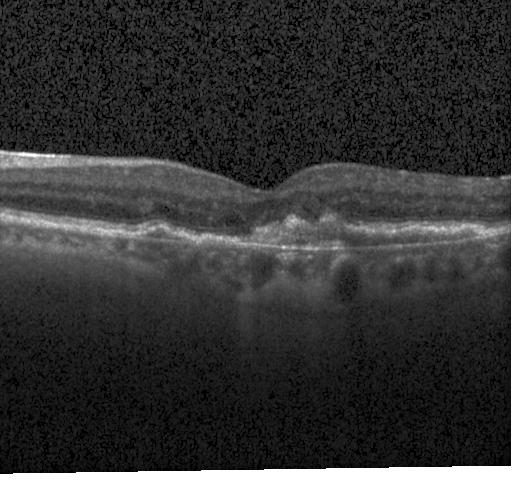

Diagnosis: choroidal neovascularization (CNV).